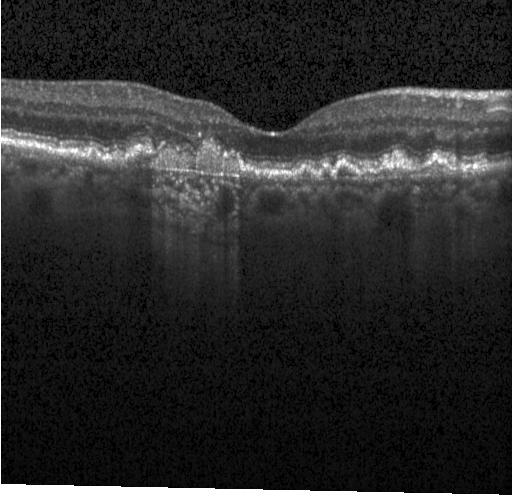
OCT line scan
Finding: a choroidal neovascular membrane.